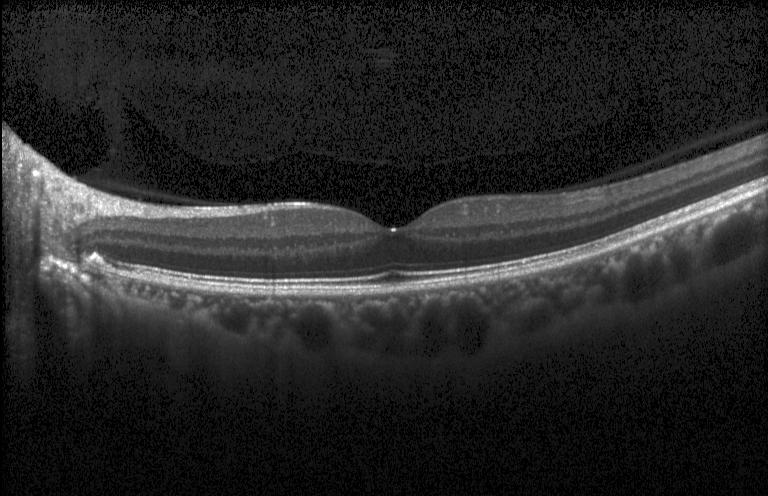 This B-scan demonstrates no choroidal neovascularization, no diabetic macular edema, and no drusen.